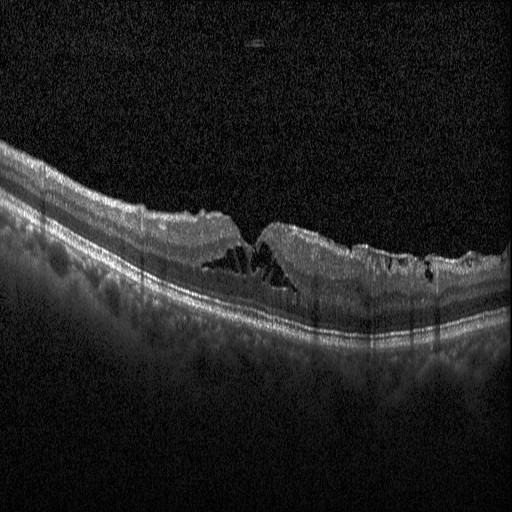
OCT B-scan, centered on the fovea — Macular OCT: diabetic macular edema (DME).